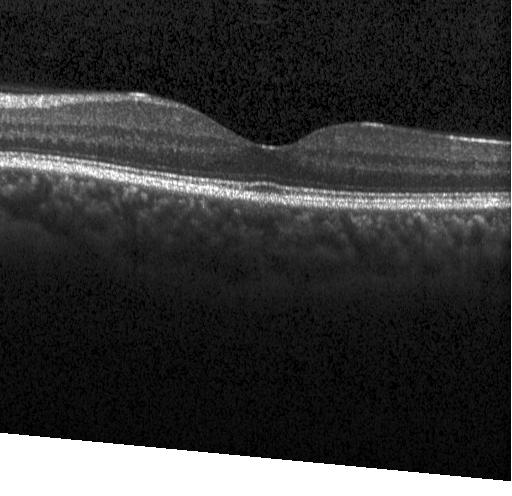 Dx: no choroidal neovascularization, no diabetic macular edema, and no drusen.